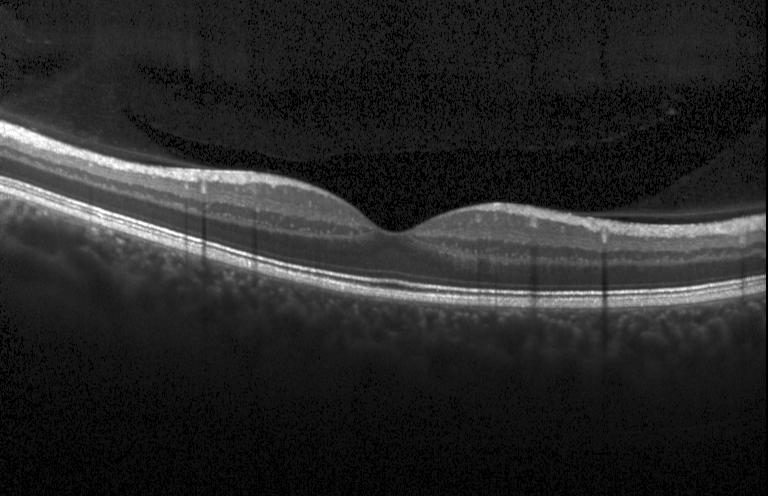

OCT B-scan, horizontal scan through the fovea, SD-OCT
Finding: no evidence of choroidal neovascularization, diabetic macular edema, or drusen.